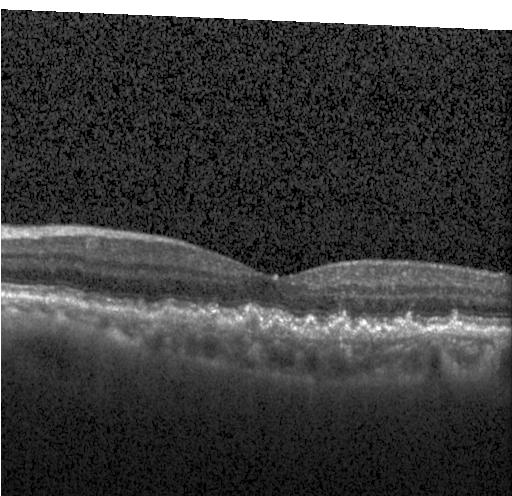
Spectral-domain optical coherence tomography · retinal OCT cross-section.
Macular OCT: sub-RPE drusenoid deposits.